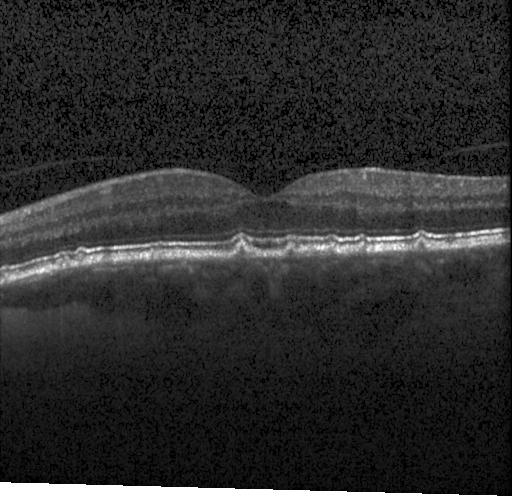 Retinal OCT cross-section.
This B-scan demonstrates sub-RPE drusenoid deposits.